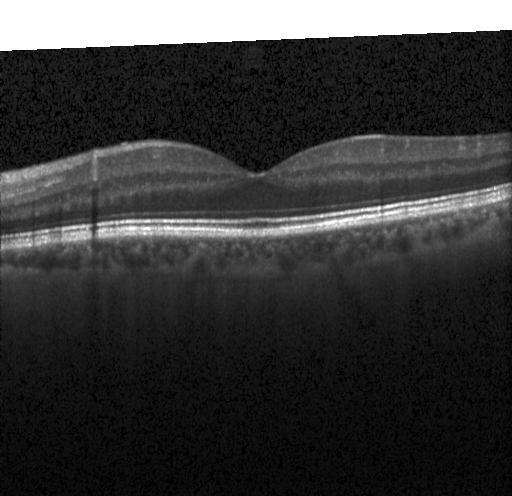

Diagnosis: no choroidal neovascularization, no diabetic macular edema, and no drusen.